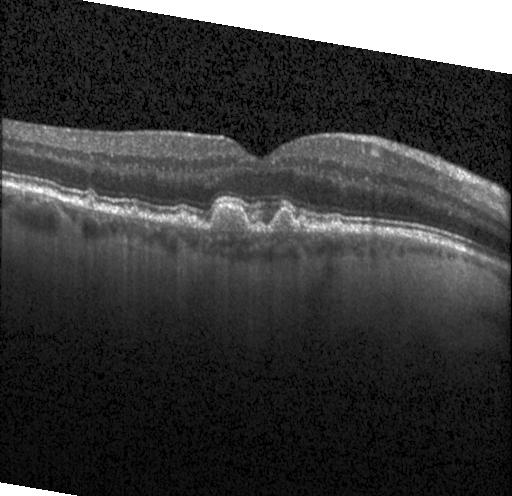 Assessment: drusen.